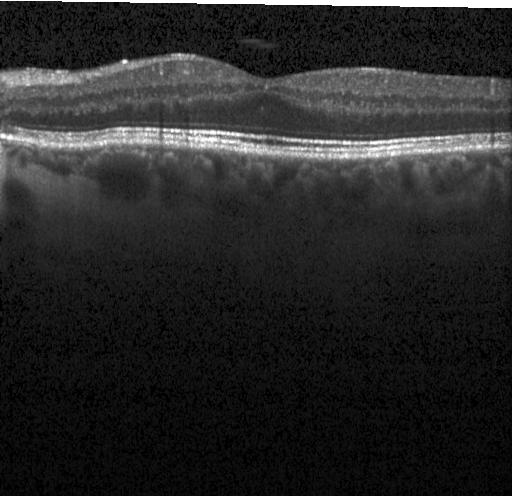 Retinal OCT cross-section showing no choroidal neovascularization, diabetic macular edema, or drusen.